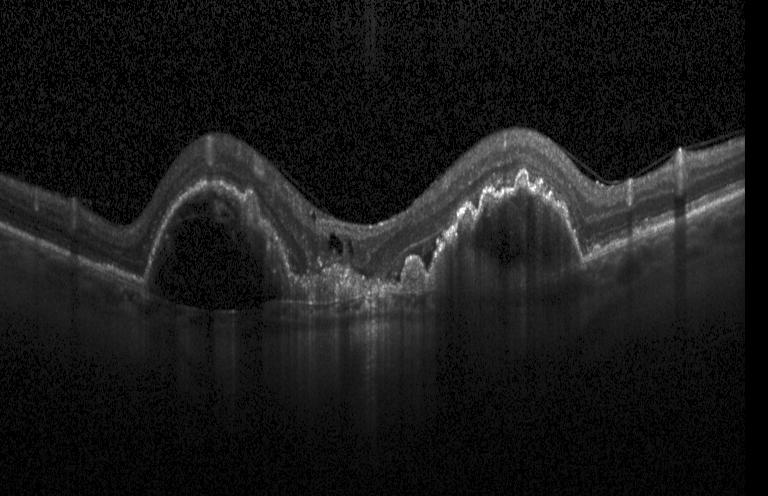
Impression: choroidal neovascularization (CNV).